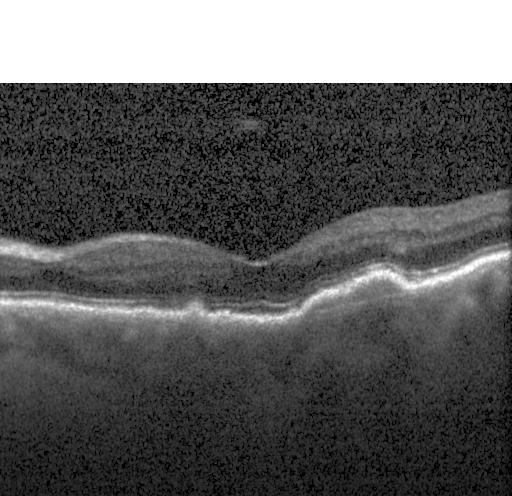
Spectral-domain OCT B-scan: choroidal neovascularization (CNV).